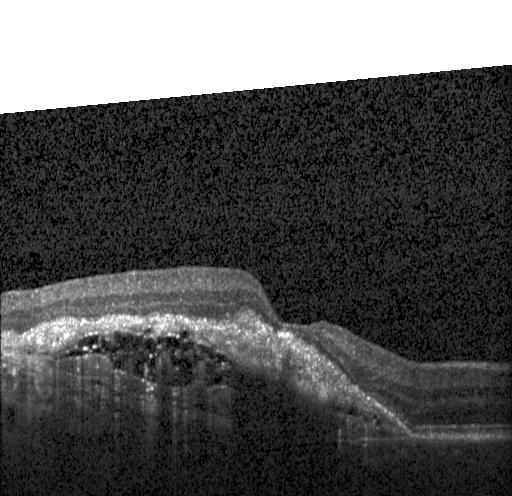
Retinal OCT B-scan; fovea-centered; acquired on a Heidelberg Spectralis; spectral-domain OCT
Diagnosis: choroidal neovascularization (CNV).